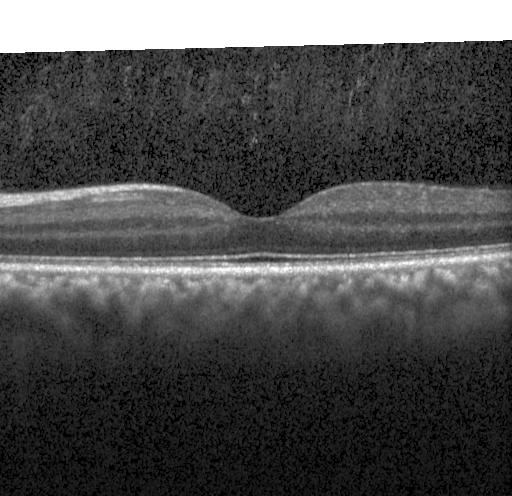 Heidelberg Spectralis, fovea-centered, OCT B-scan, spectral-domain optical coherence tomography.
Diagnosis: no choroidal neovascularization, diabetic macular edema, or drusen.